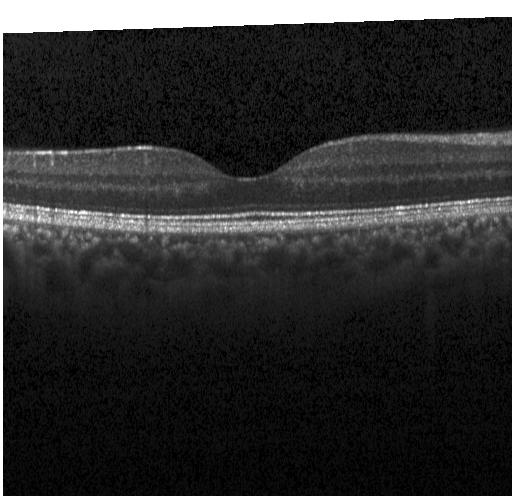
Retinal OCT cross-section.
The scan shows no choroidal neovascularization, diabetic macular edema, or drusen.